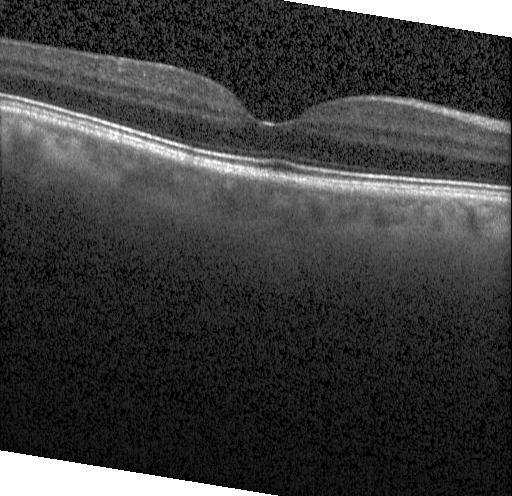
OCT line scan
Impression: no choroidal neovascularization, diabetic macular edema, or drusen.